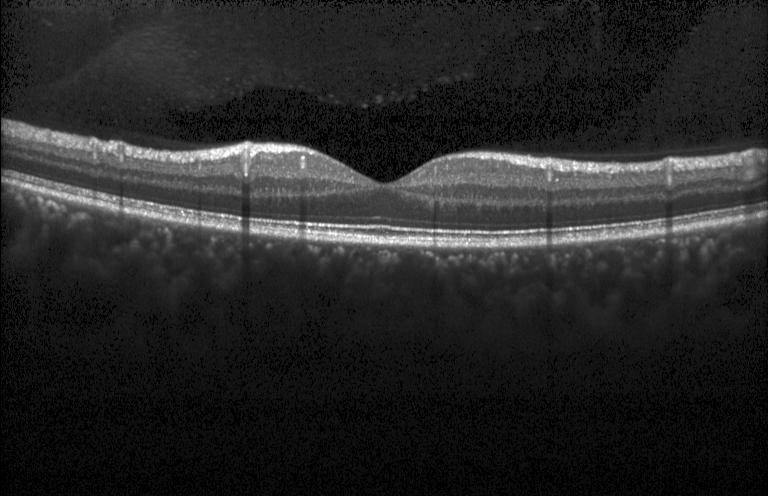 OCT B-scan. Macular OCT: no choroidal neovascularization, diabetic macular edema, or drusen.